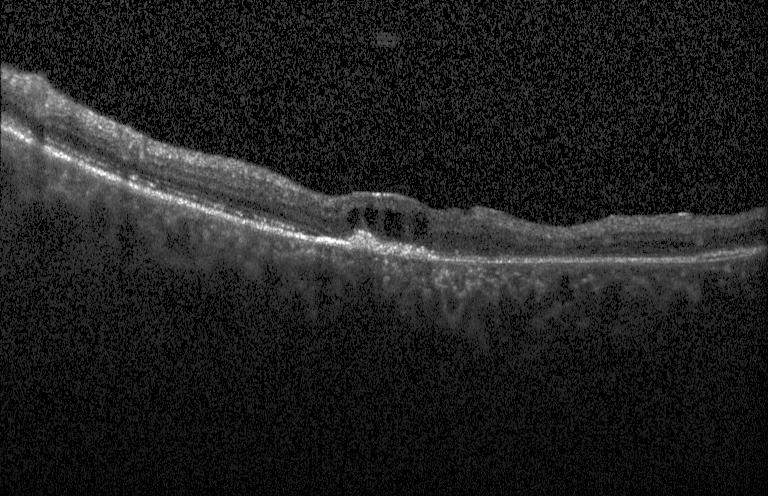
The scan shows a choroidal neovascular membrane.